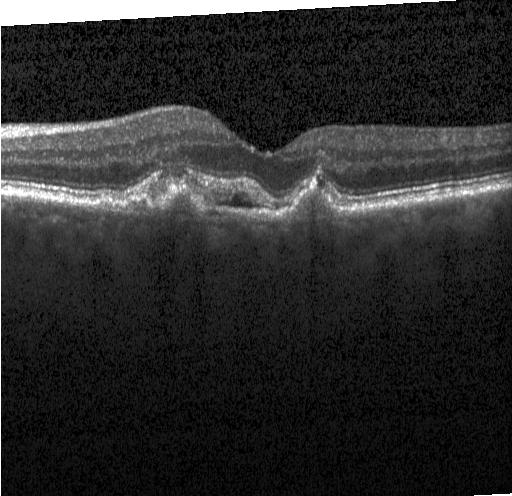
OCT finding: a choroidal neovascular membrane.